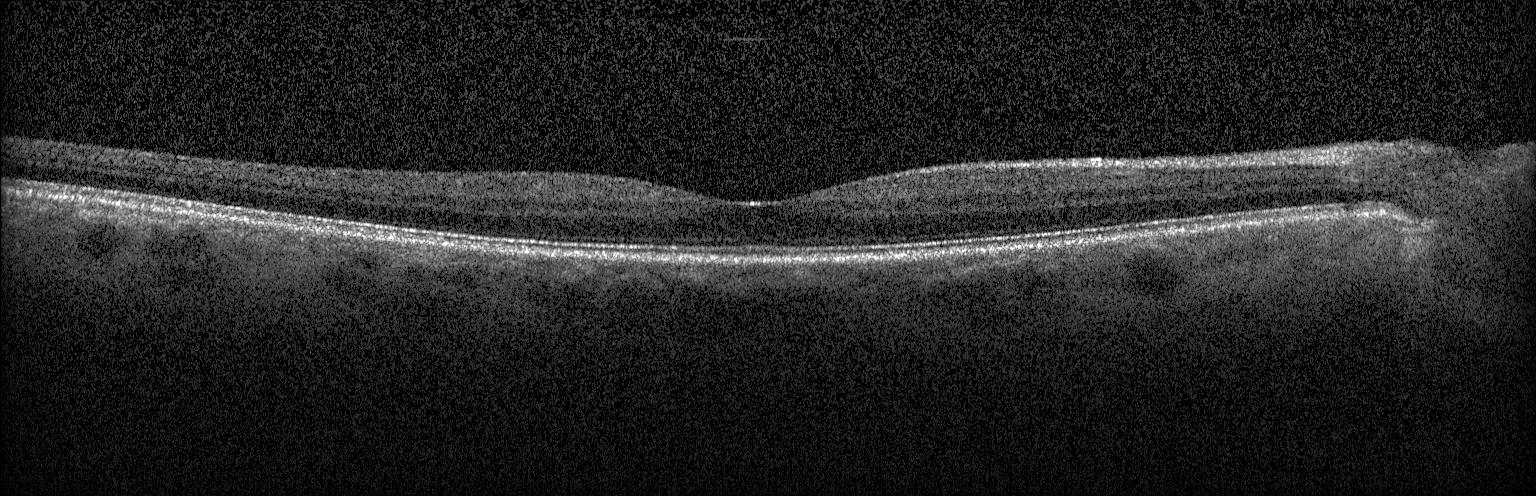

Diagnosis: no choroidal neovascularization, diabetic macular edema, or drusen.